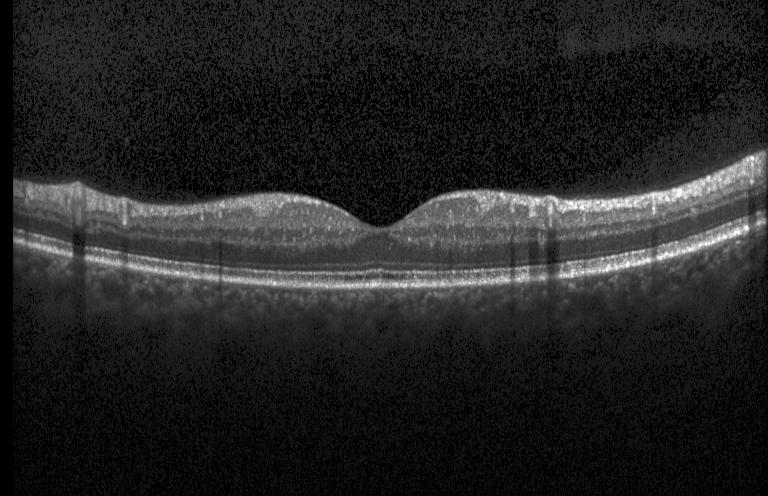
Spectral-domain optical coherence tomography; retinal OCT cross-section; Heidelberg Spectralis.
Assessment: no evidence of CNV, DME, or drusen.